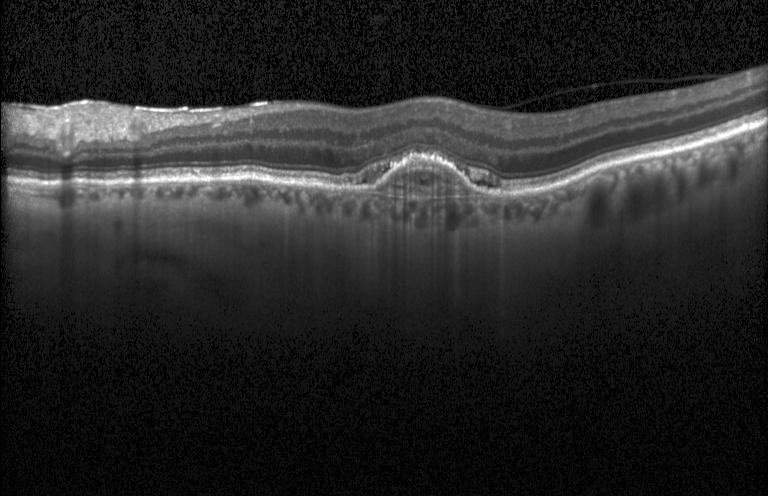
Heidelberg Spectralis. Macular scan. OCT B-scan. SD-OCT. Diagnosis: a choroidal neovascular membrane.